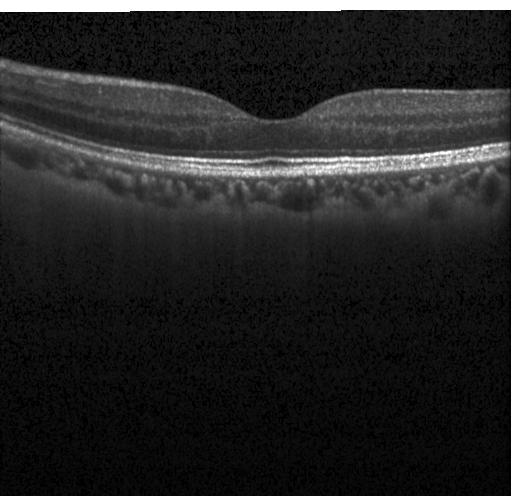 Macular OCT demonstrating no choroidal neovascularization, no diabetic macular edema, and no drusen.